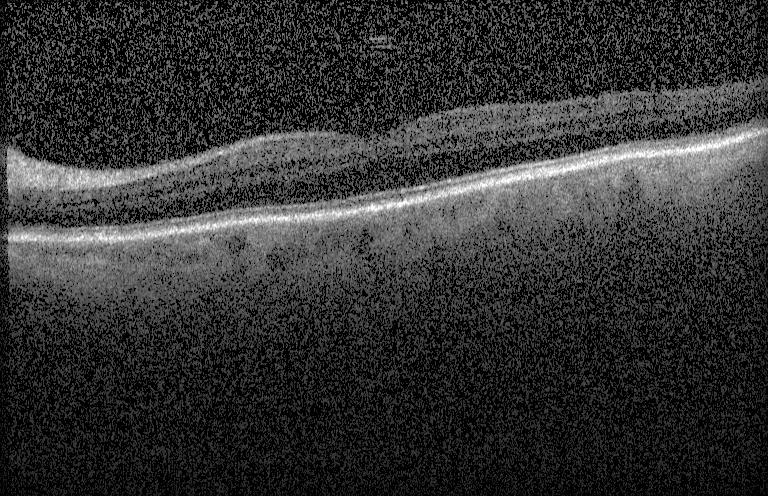

Optical coherence tomography scan, spectral-domain OCT — This B-scan demonstrates no evidence of choroidal neovascularization, diabetic macular edema, or drusen.